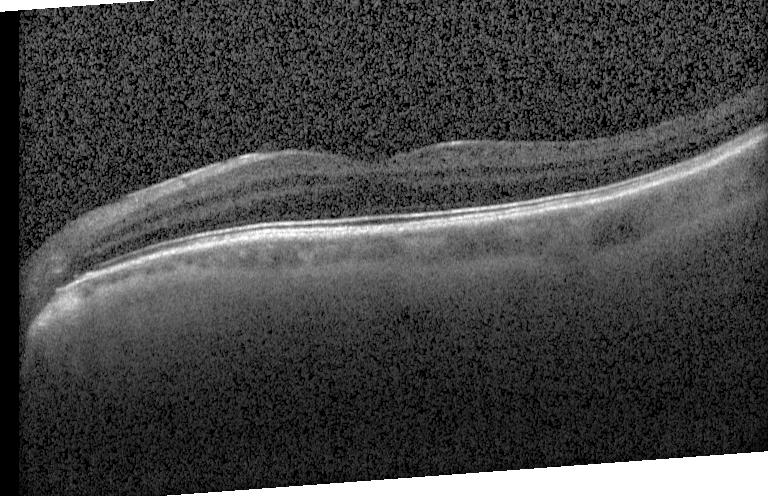
Optical coherence tomography B-scan; Heidelberg Spectralis OCT system
Impression: no evidence of choroidal neovascularization, diabetic macular edema, or drusen.